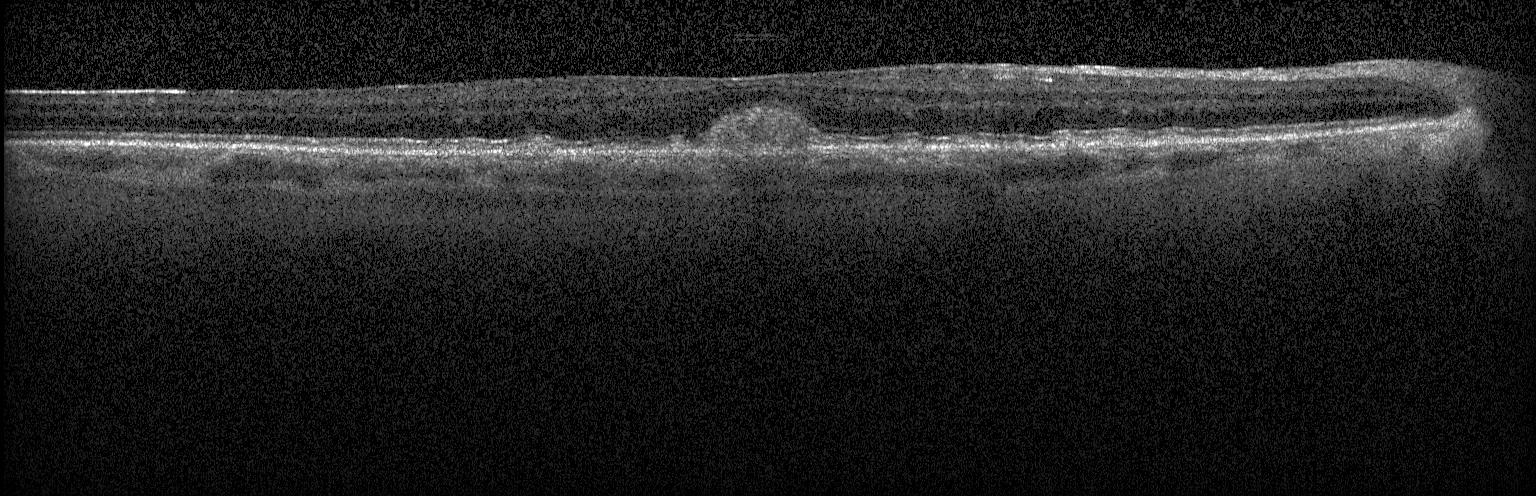 Heidelberg Spectralis OCT system. Optical coherence tomography B-scan — This B-scan demonstrates CNV.